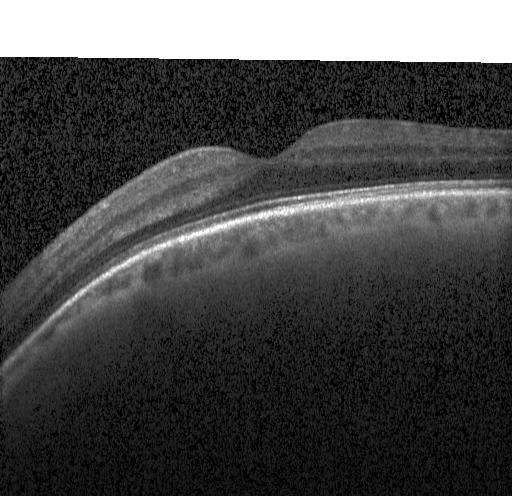 OCT B-scan; spectral-domain OCT; horizontal scan through the fovea. Finding: neither choroidal neovascularization, diabetic macular edema, nor drusen.